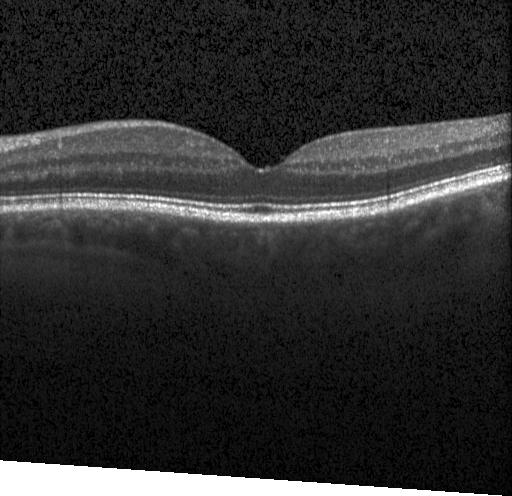

Finding: no choroidal neovascularization, diabetic macular edema, or drusen.